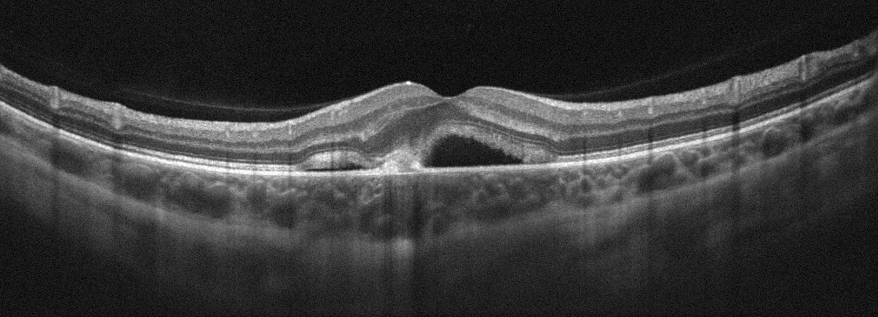

Retinal OCT B-scan.
Impression: age-related macular degeneration (AMD).